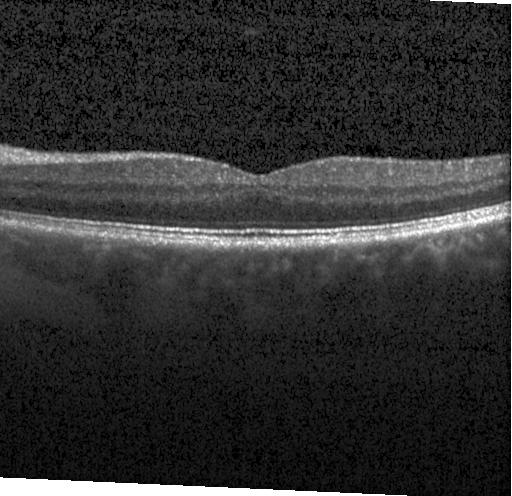
Macular scan · OCT B-scan — Macular OCT: no choroidal neovascularization, diabetic macular edema, or drusen.